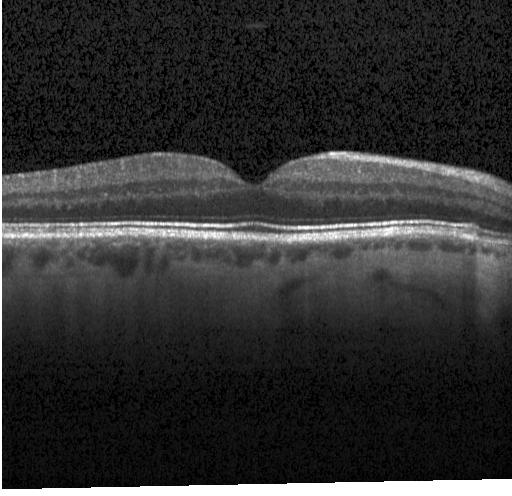
Spectral-domain optical coherence tomography, instrument: Heidelberg Spectralis, retinal OCT cross-section — Impression: no evidence of CNV, DME, or drusen.